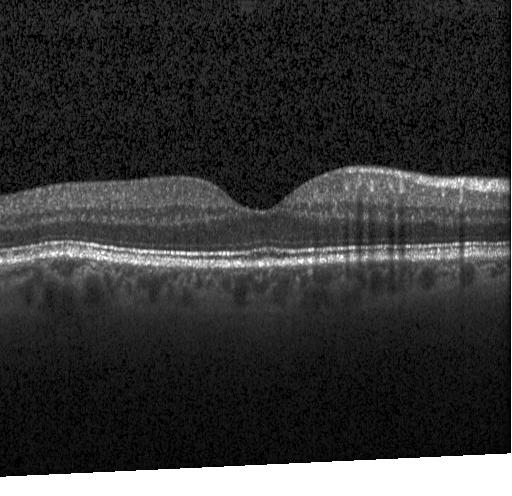
Spectral-domain OCT. Horizontal scan through the fovea. Retinal OCT B-scan — No choroidal neovascularization, no diabetic macular edema, and no drusen.